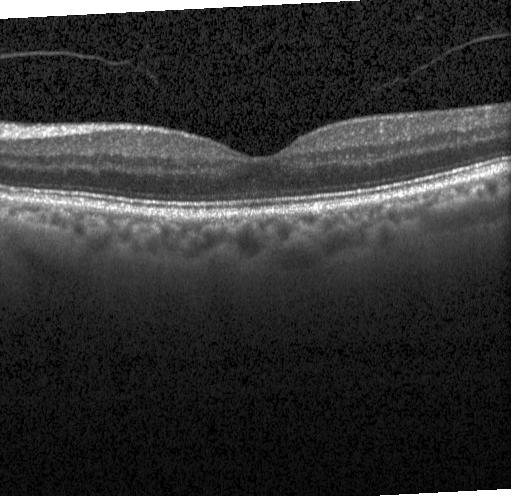
OCT B-scan
Impression: neither choroidal neovascularization, diabetic macular edema, nor drusen.